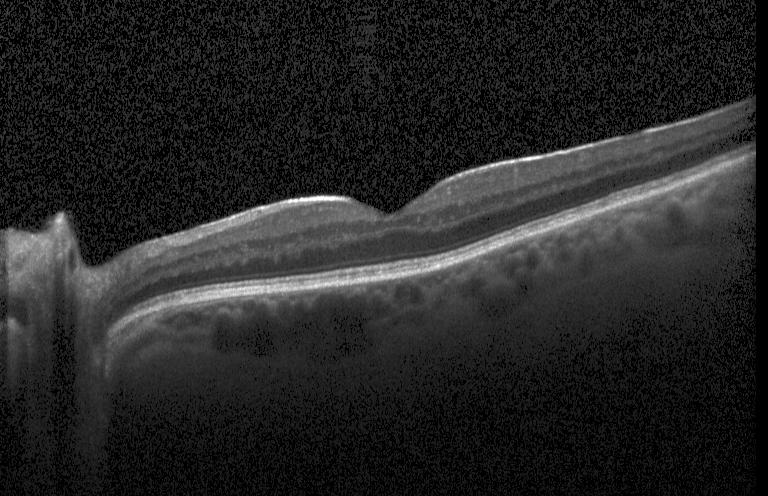 Optical coherence tomography scan.
Macular OCT: neither choroidal neovascularization, diabetic macular edema, nor drusen.